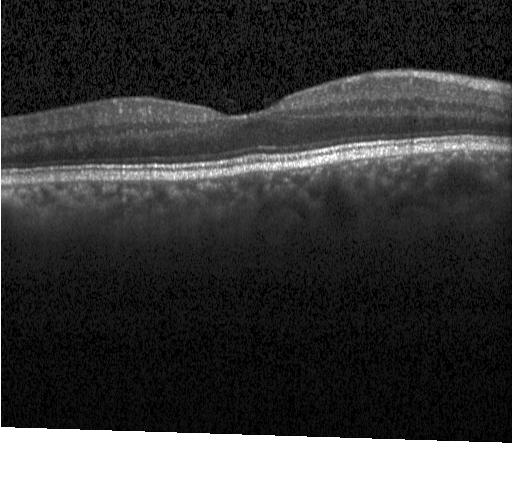 Retinal OCT cross-section. Heidelberg Spectralis. Through the macula. Spectral-domain optical coherence tomography — This B-scan demonstrates no choroidal neovascularization, diabetic macular edema, or drusen.